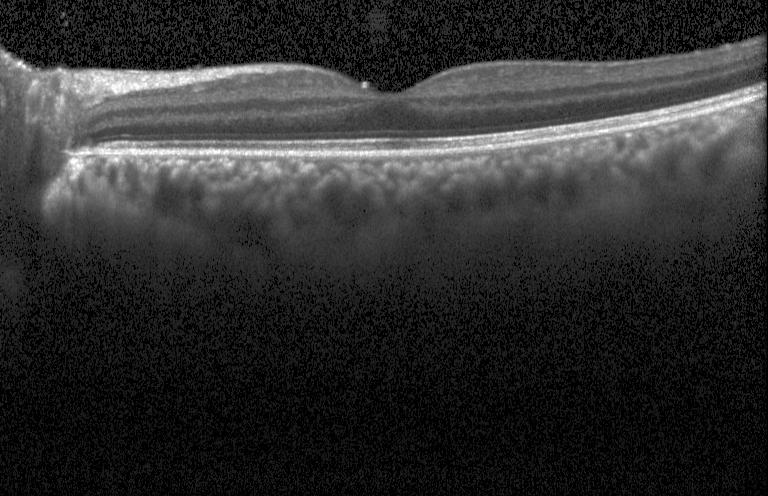 Retinal OCT B-scan — Impression: no choroidal neovascularization, no diabetic macular edema, and no drusen.